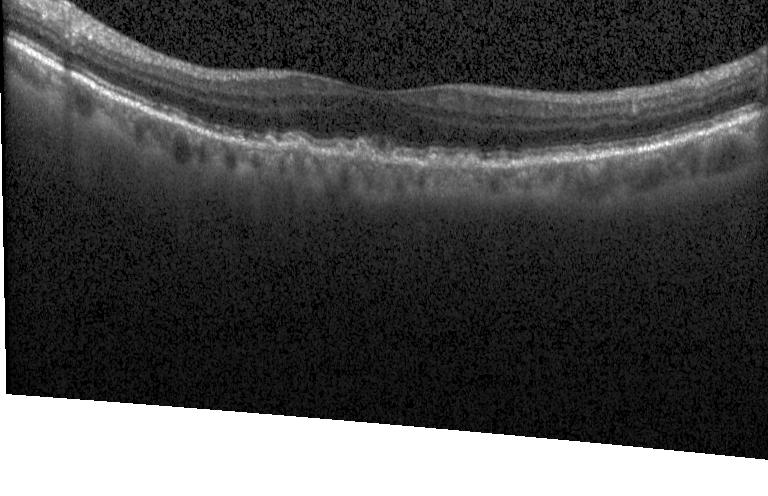
Macular scan; OCT B-scan; SD-OCT — Assessment: drusen.